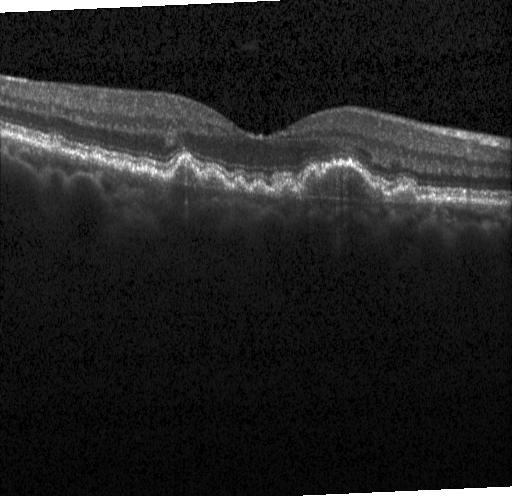
Sub-RPE drusenoid deposits.